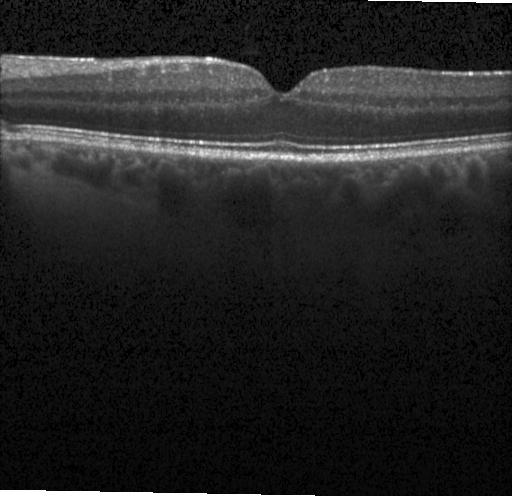
Optical coherence tomography scan · fovea-centered. Diagnosis: no choroidal neovascularization, no diabetic macular edema, and no drusen.